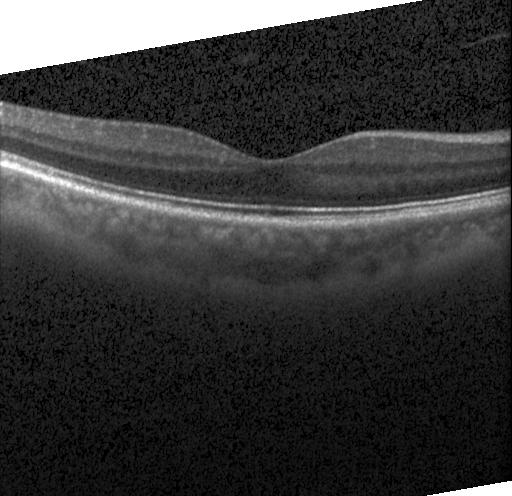

OCT B-scan, through the macula.
Diagnosis: no choroidal neovascularization, no diabetic macular edema, and no drusen.